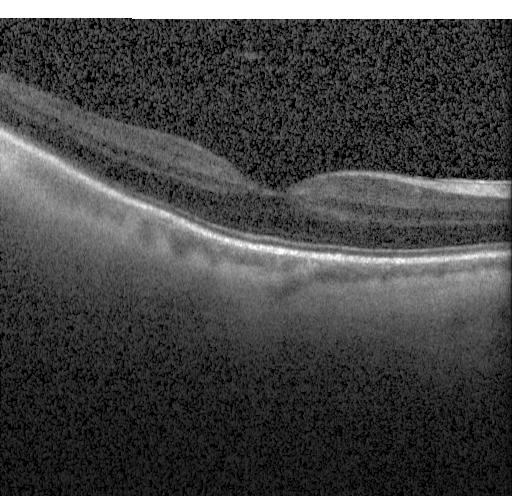
OCT line scan, Heidelberg Spectralis, horizontal scan through the fovea. The scan shows no choroidal neovascularization, diabetic macular edema, or drusen.